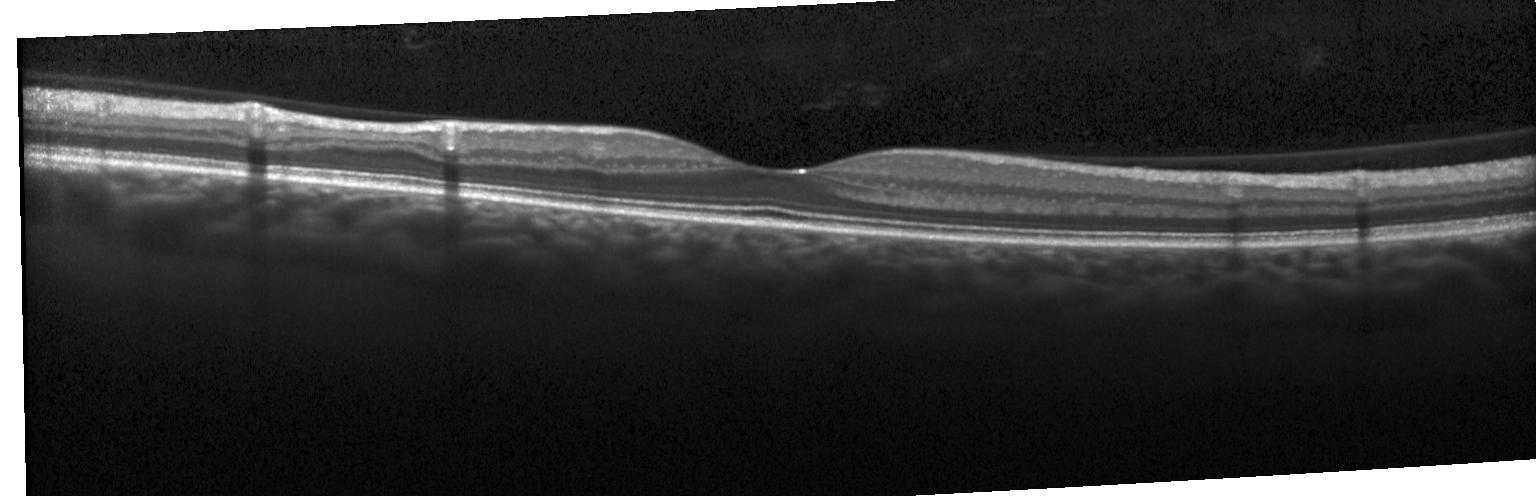
Optical coherence tomography scan
Assessment: neither choroidal neovascularization, diabetic macular edema, nor drusen.